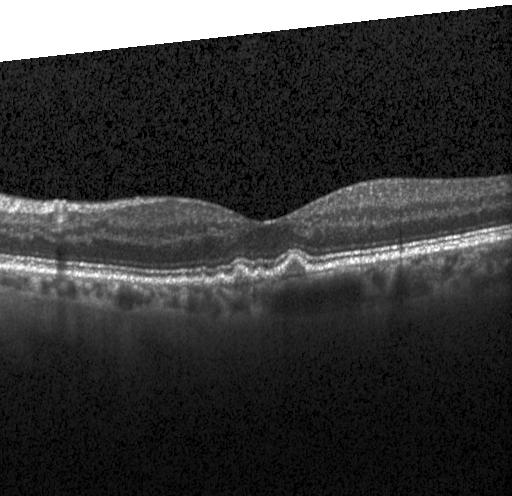 Assessment: multiple drusen.